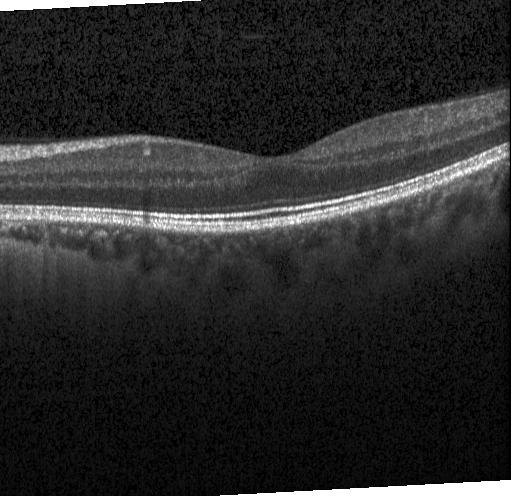
Neither CNV, DME, nor drusen.